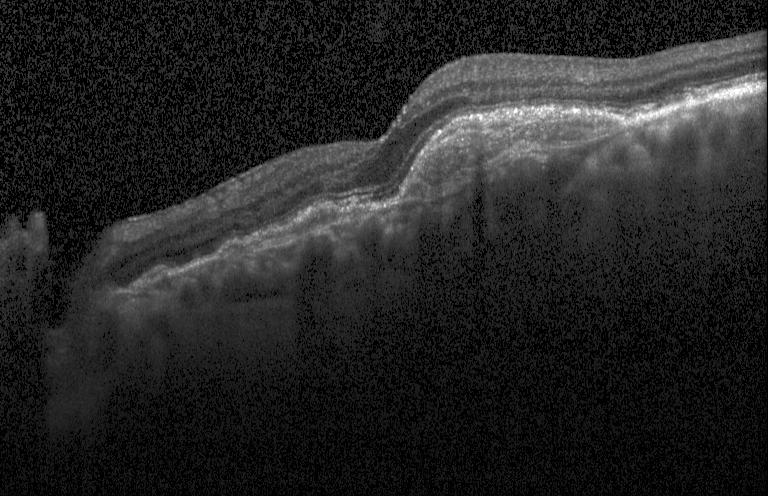

Impression: choroidal neovascularization.